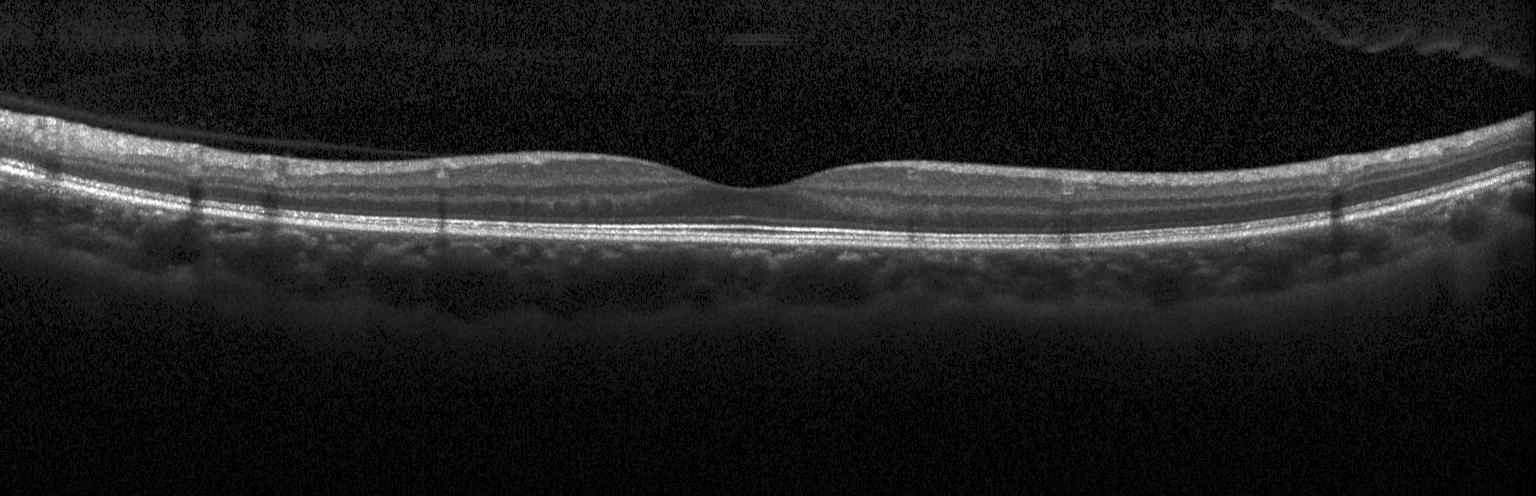

OCT line scan — Impression: no evidence of choroidal neovascularization, diabetic macular edema, or drusen.